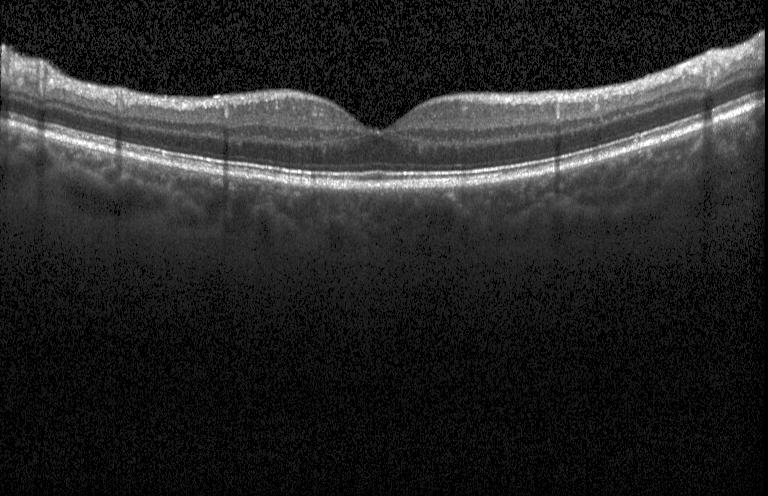

Dx: no evidence of choroidal neovascularization, diabetic macular edema, or drusen.